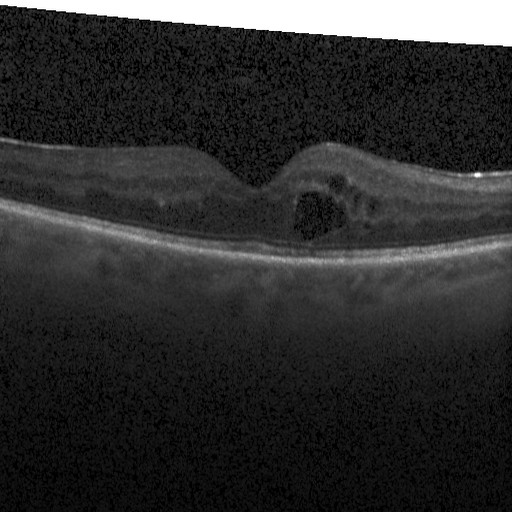 Spectral-domain OCT B-scan: diabetic macular edema (DME).